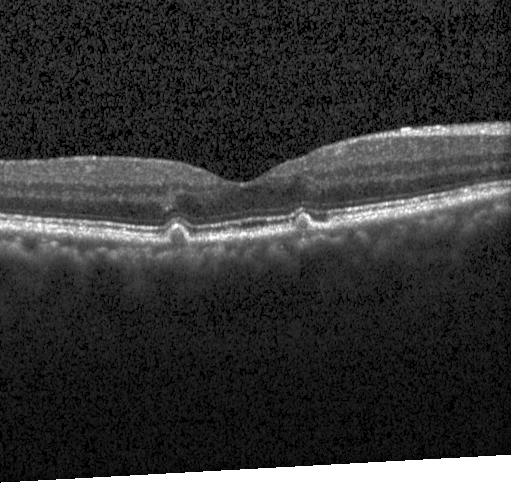

Spectral-domain optical coherence tomography · fovea-centered · optical coherence tomography B-scan · Heidelberg Spectralis OCT system.
Drusen.